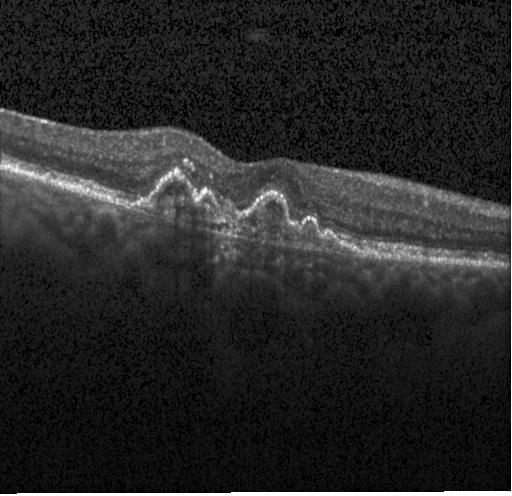

OCT finding: a choroidal neovascular membrane.